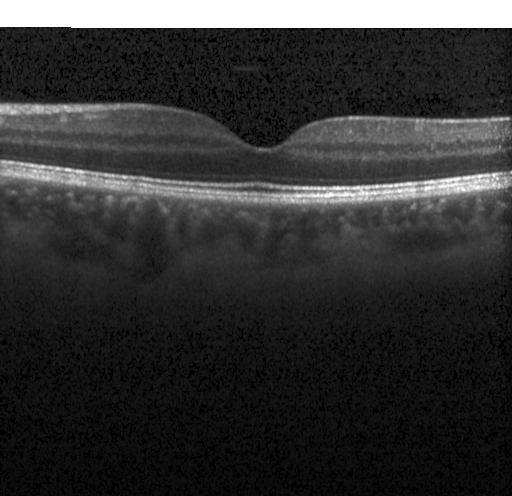 Optical coherence tomography B-scan; SD-OCT; Heidelberg Spectralis — Impression: no choroidal neovascularization, no diabetic macular edema, and no drusen.